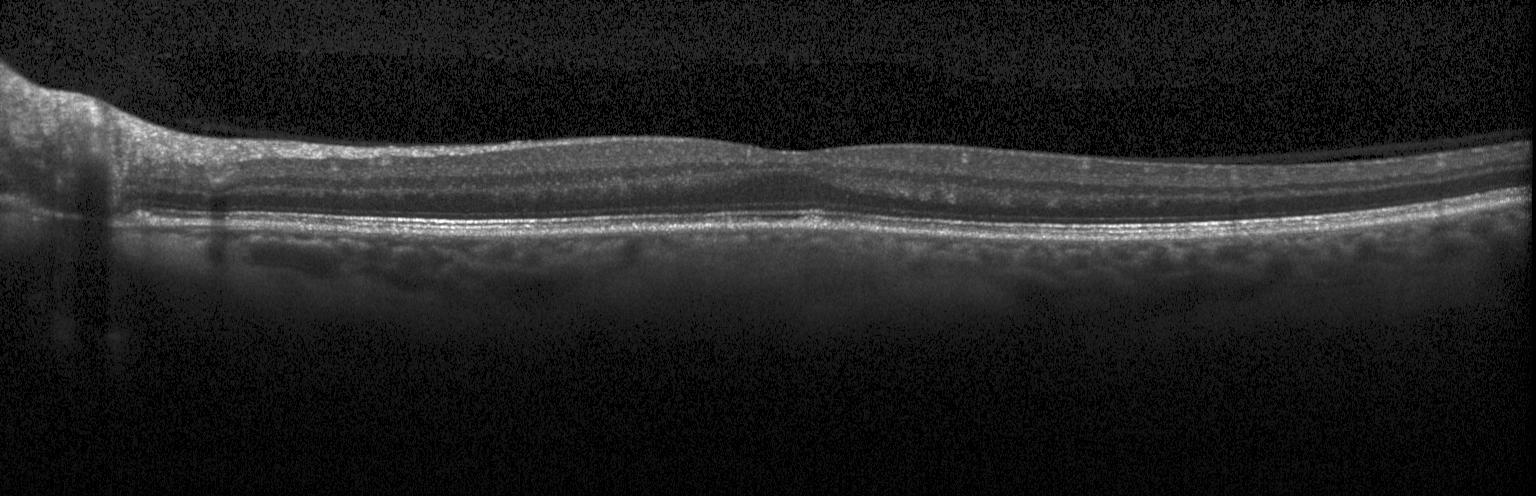

Heidelberg Spectralis OCT system · retinal OCT cross-section — The scan shows no choroidal neovascularization, no diabetic macular edema, and no drusen.